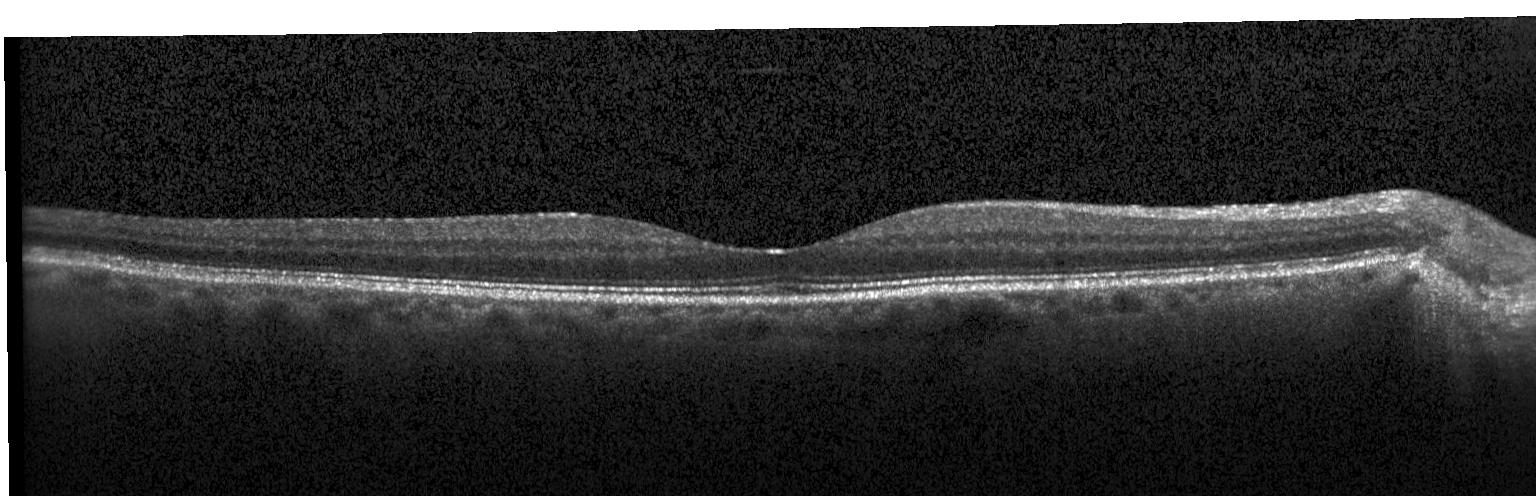

Optical coherence tomography B-scan. SD-OCT. Centered on the fovea — No choroidal neovascularization, no diabetic macular edema, and no drusen.